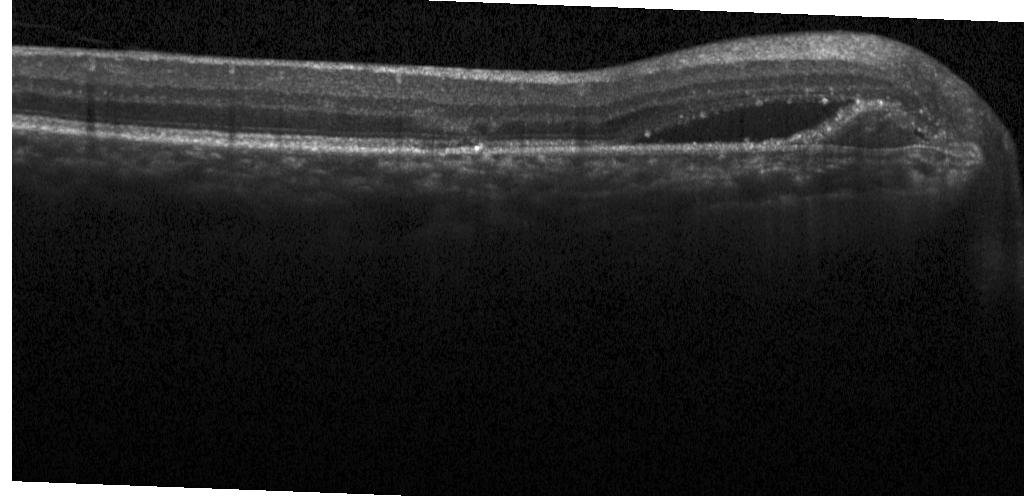 Spectral-domain OCT B-scan: choroidal neovascularization (CNV).